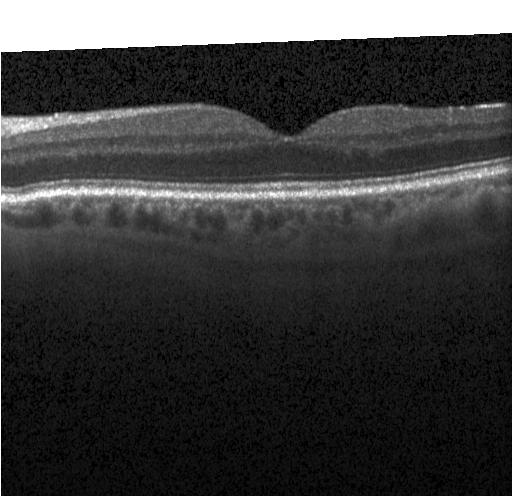
Optical coherence tomography B-scan.
Impression: neither CNV, DME, nor drusen.